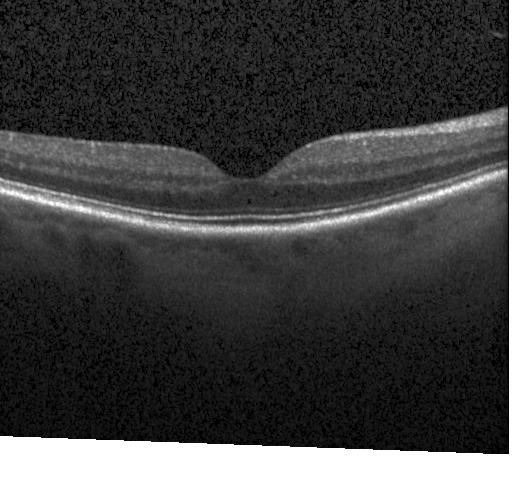

Spectral-domain OCT B-scan: no evidence of choroidal neovascularization, diabetic macular edema, or drusen.